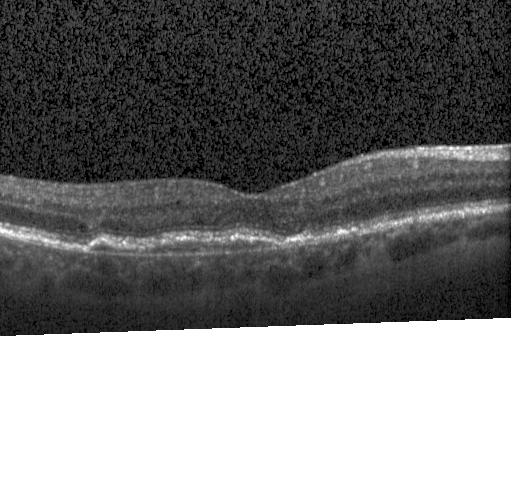

Retinal OCT B-scan. Spectral-domain optical coherence tomography. Macular scan
Diagnosis: choroidal neovascularization.